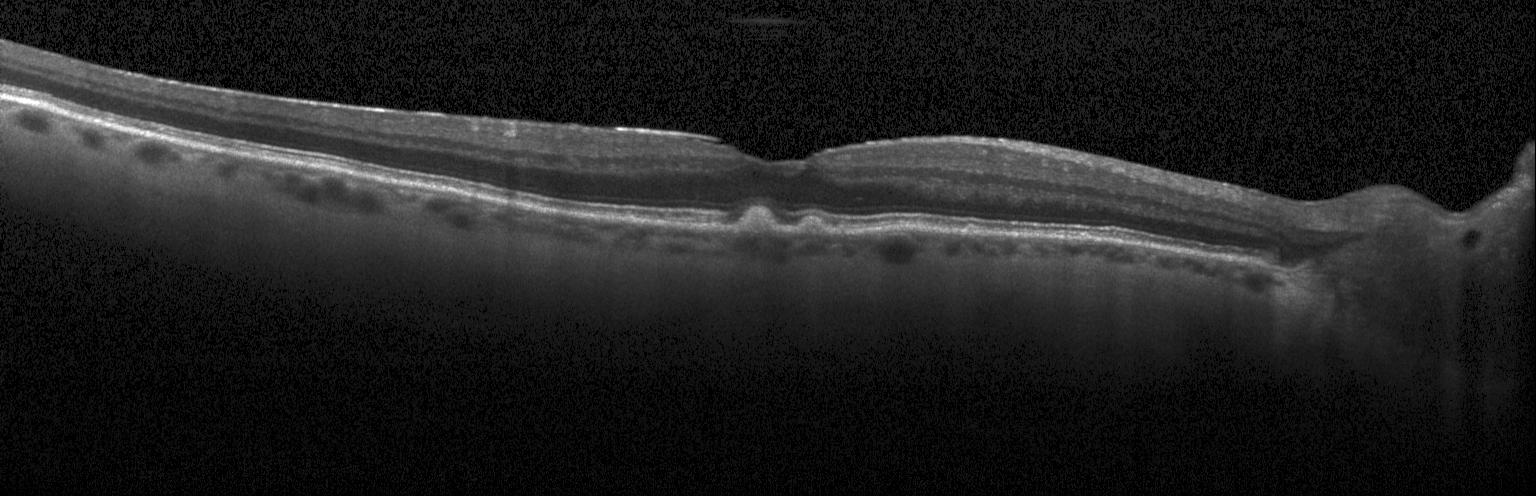 Acquired on a Heidelberg Spectralis; retinal OCT B-scan; spectral-domain OCT.
Diagnosis: sub-RPE drusenoid deposits.